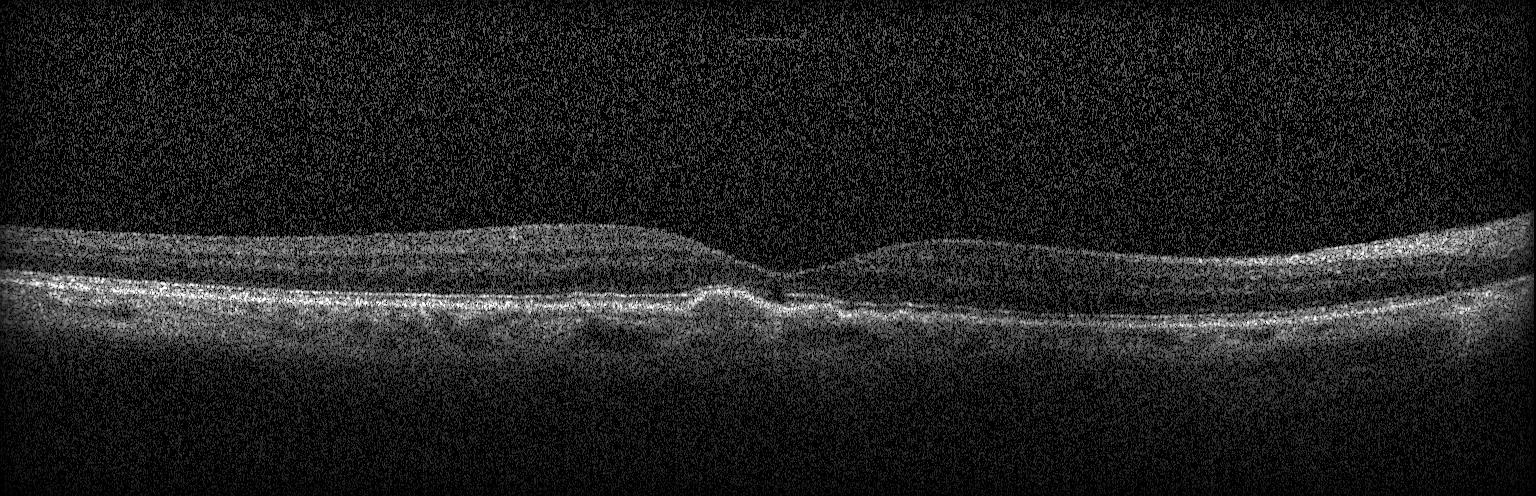
OCT finding: sub-RPE drusenoid deposits.